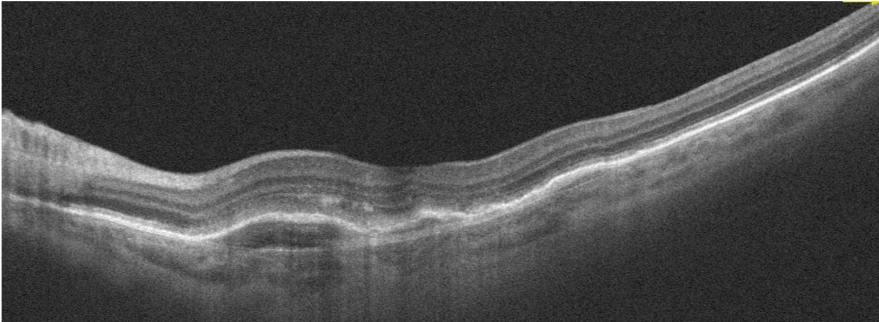

Optical coherence tomography B-scan. Age-related macular degeneration (AMD).